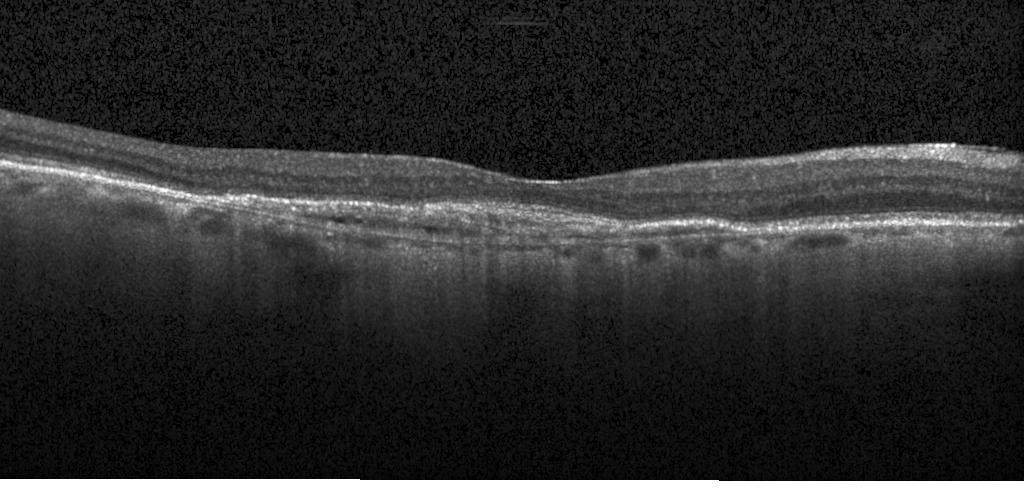
Macular OCT demonstrating choroidal neovascularization (CNV).